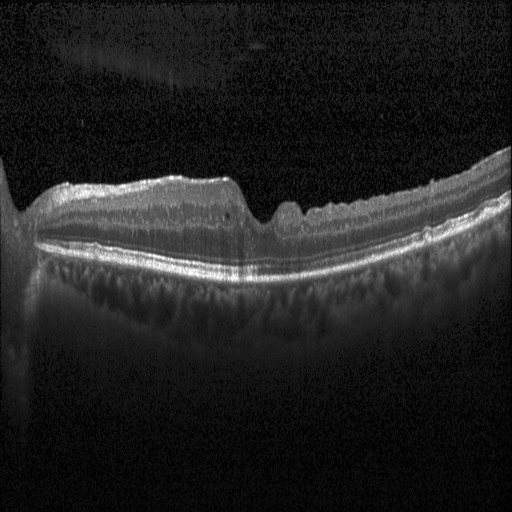
Spectral-domain OCT B-scan: diabetic macular edema.